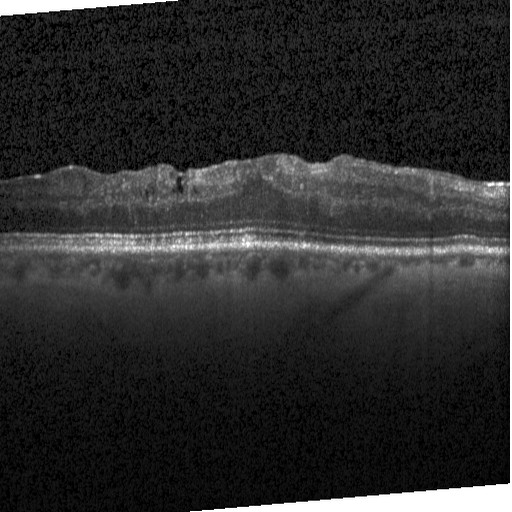

OCT scan showing diabetic macular edema.